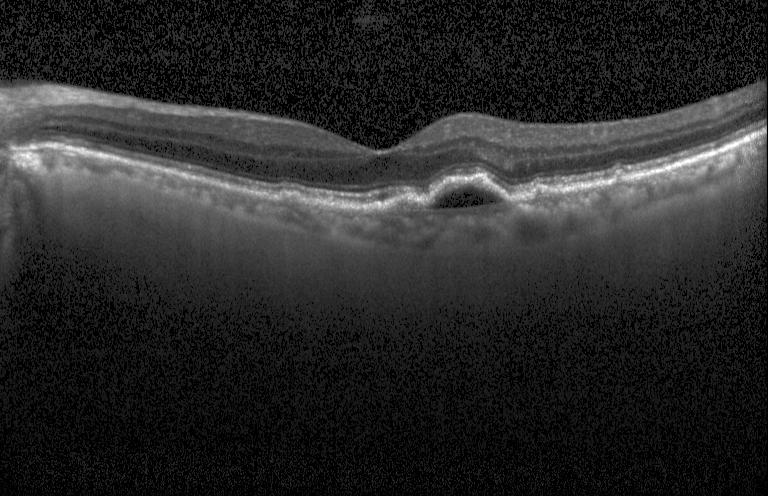

Diagnosis: CNV.